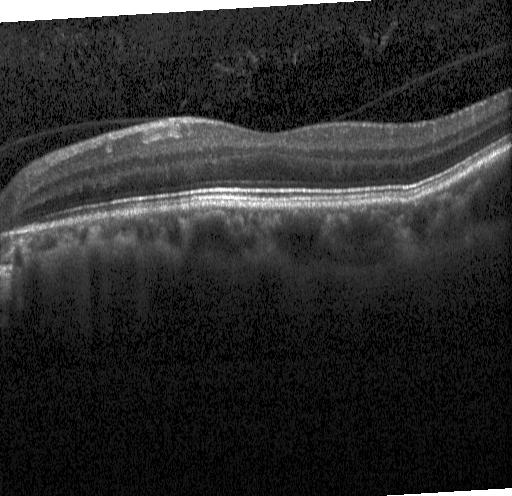 Macular OCT: no choroidal neovascularization, diabetic macular edema, or drusen.